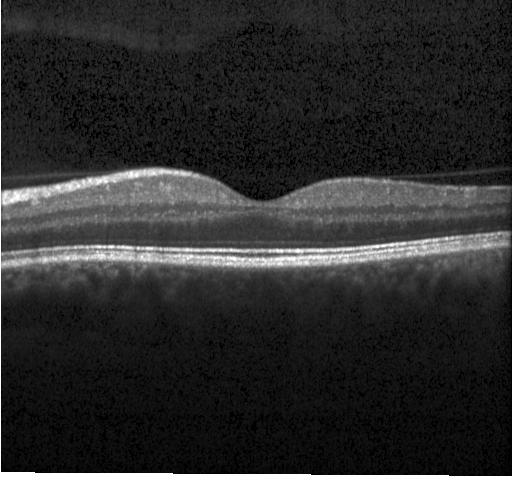

Acquired on a Heidelberg Spectralis. Spectral-domain OCT. Fovea-centered. Optical coherence tomography scan.
Diagnosis: neither choroidal neovascularization, diabetic macular edema, nor drusen.